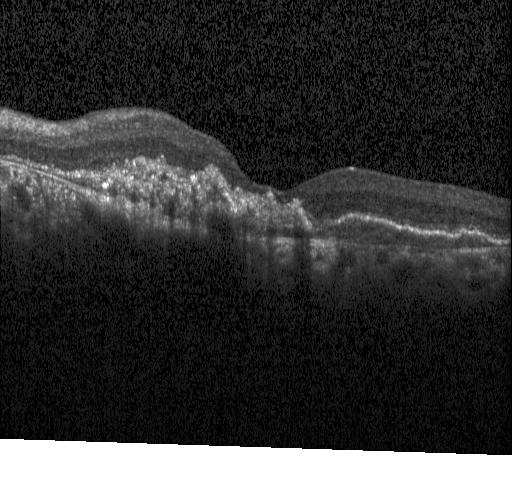 This B-scan demonstrates a choroidal neovascular membrane.